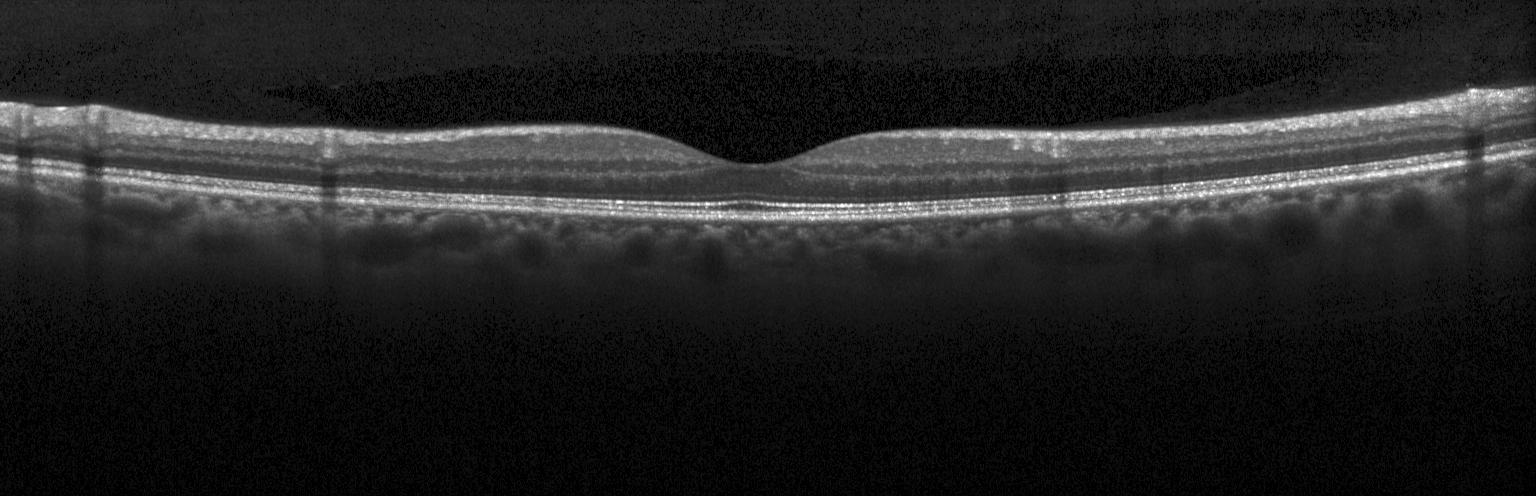

Retinal OCT B-scan · macular scan
Finding: neither choroidal neovascularization, diabetic macular edema, nor drusen.